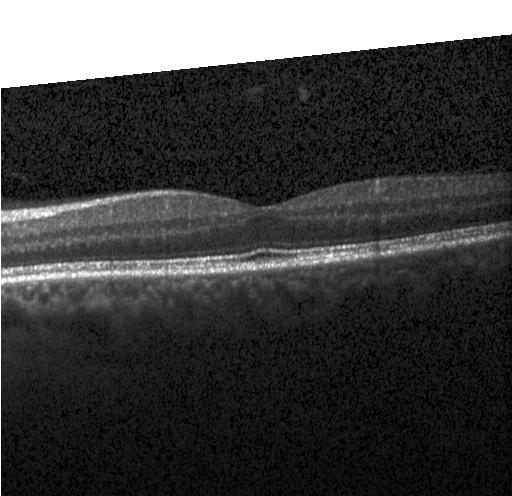

Macular OCT demonstrating neither CNV, DME, nor drusen.